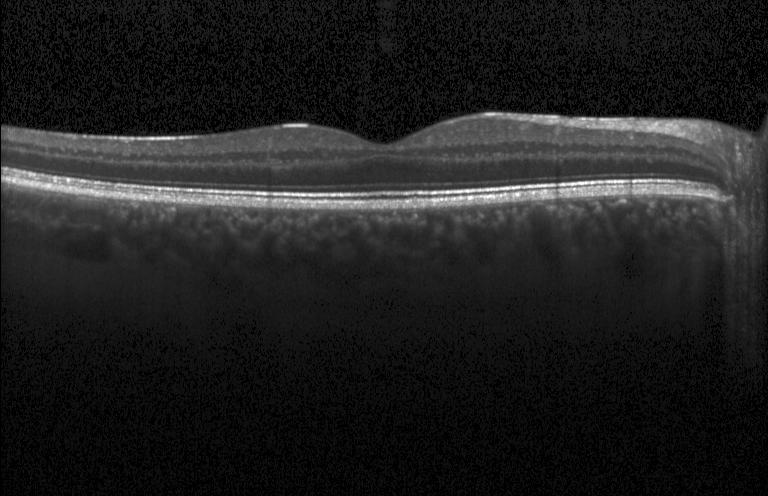
Horizontal scan through the fovea. Optical coherence tomography scan. This B-scan demonstrates no evidence of CNV, DME, or drusen.